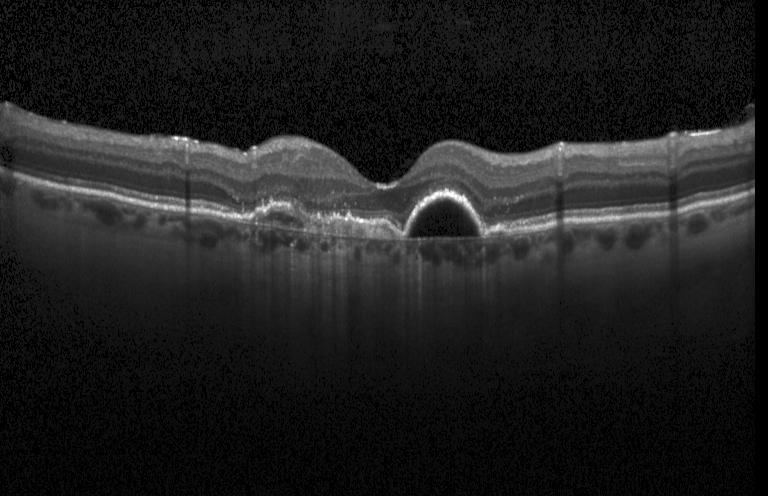
OCT finding: choroidal neovascularization (CNV).